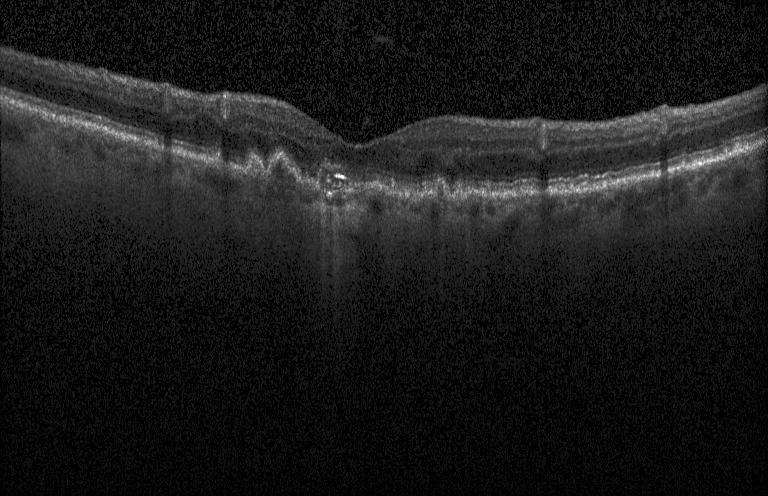 OCT line scan, Heidelberg Spectralis OCT system, spectral-domain OCT, macular scan. Finding: multiple drusen.